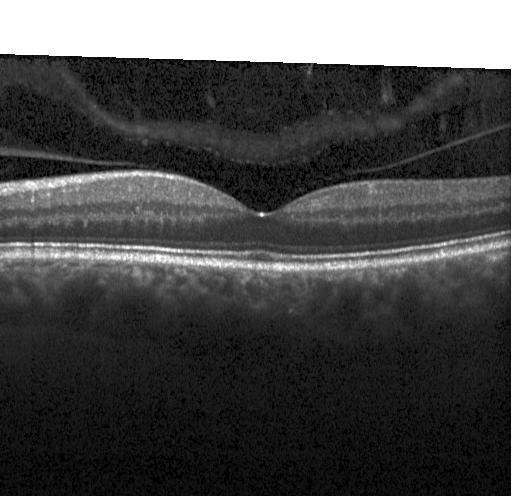 Optical coherence tomography scan; Heidelberg Spectralis; spectral-domain OCT; through the macula — Neither choroidal neovascularization, diabetic macular edema, nor drusen.